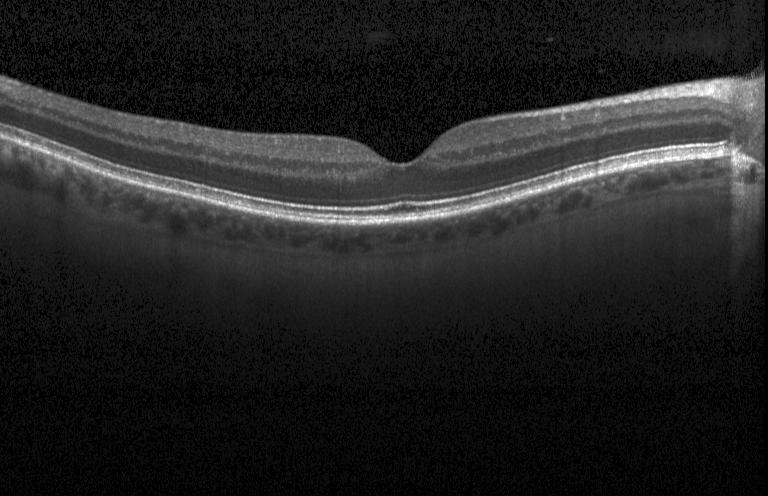
OCT scan showing no choroidal neovascularization, diabetic macular edema, or drusen.